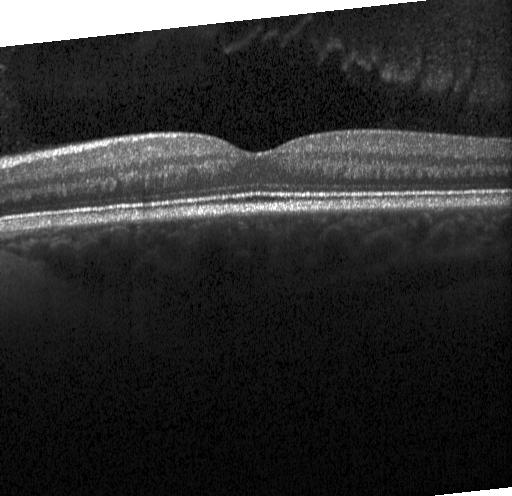 Retinal OCT B-scan
Impression: no CNV, DME, or drusen.